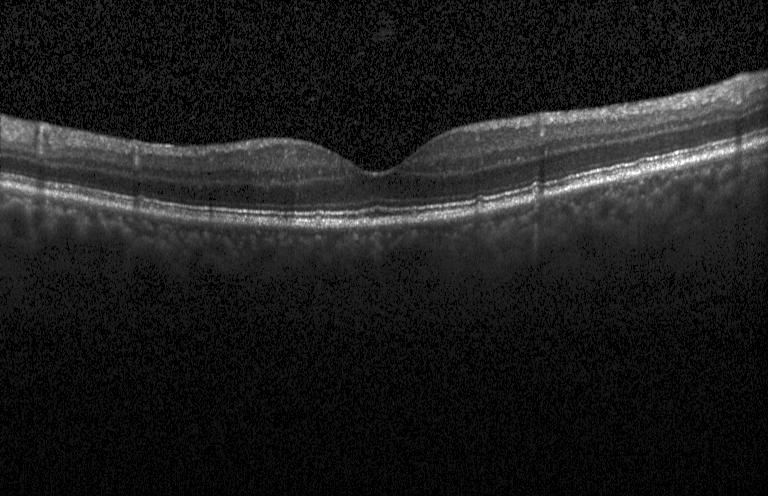
Retinal OCT cross-section. Multiple drusen.